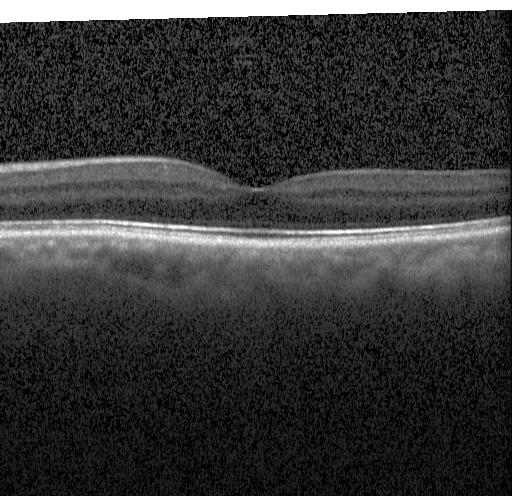 Retinal OCT cross-section showing no evidence of choroidal neovascularization, diabetic macular edema, or drusen.